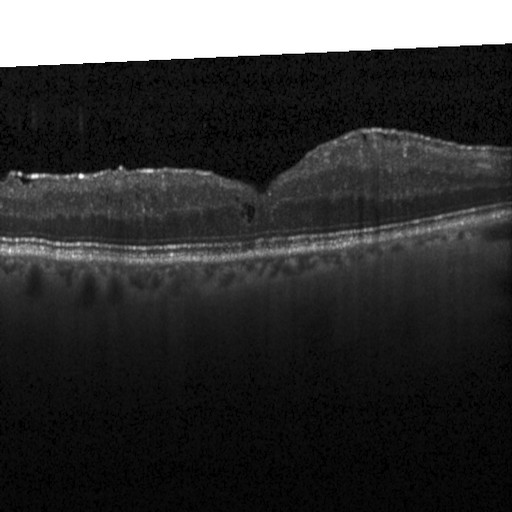

Diagnosis: diabetic macular edema.